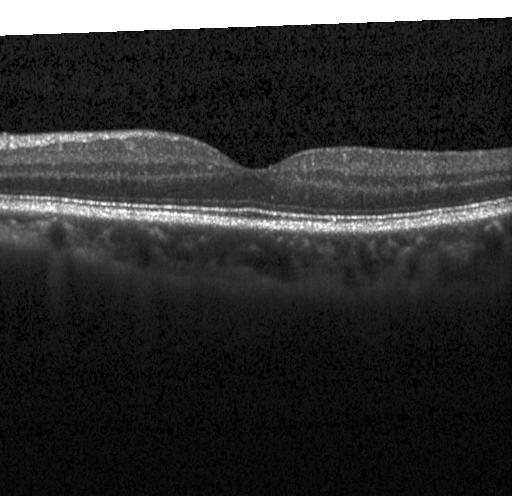
Impression: neither CNV, DME, nor drusen.